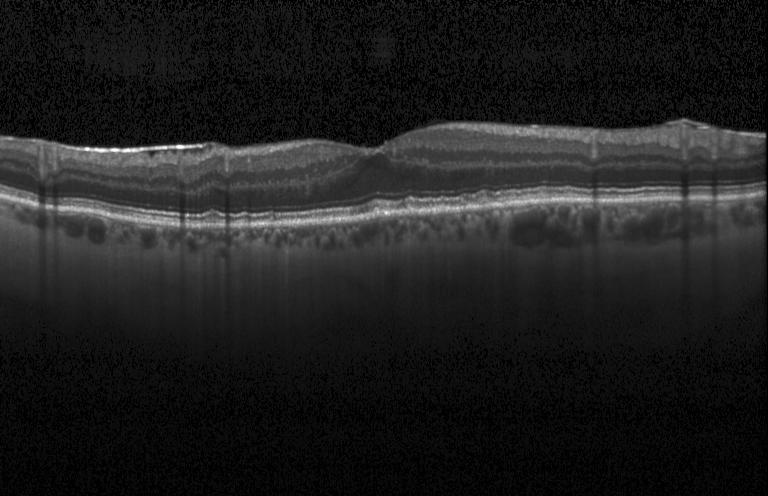 Sub-RPE drusenoid deposits.